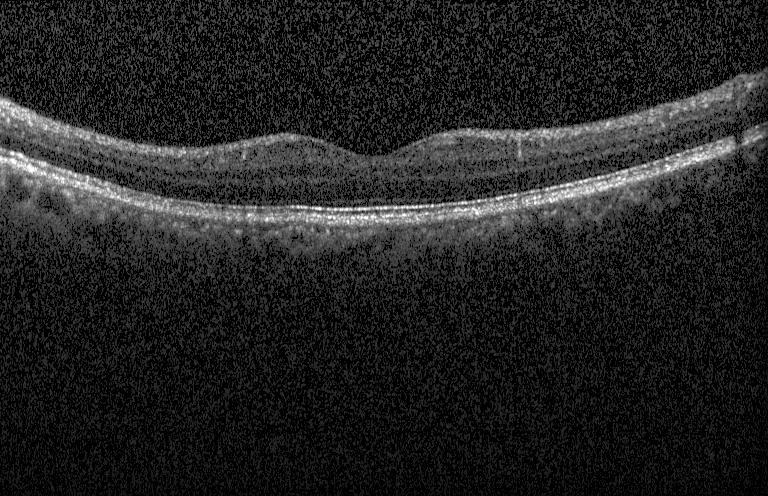

Retinal OCT cross-section. Centered on the fovea.
No evidence of choroidal neovascularization, diabetic macular edema, or drusen.